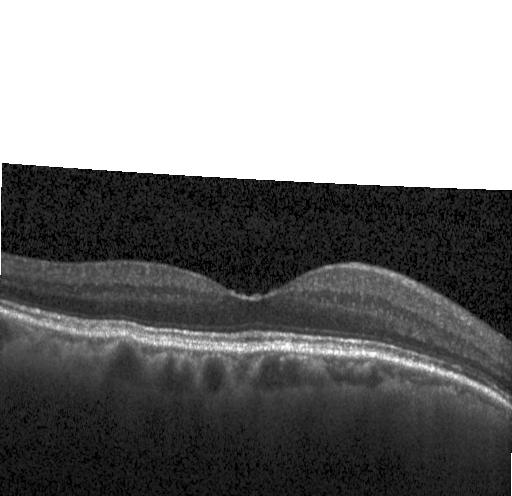
Optical coherence tomography scan; centered on the fovea.
Diagnosis: no evidence of choroidal neovascularization, diabetic macular edema, or drusen.